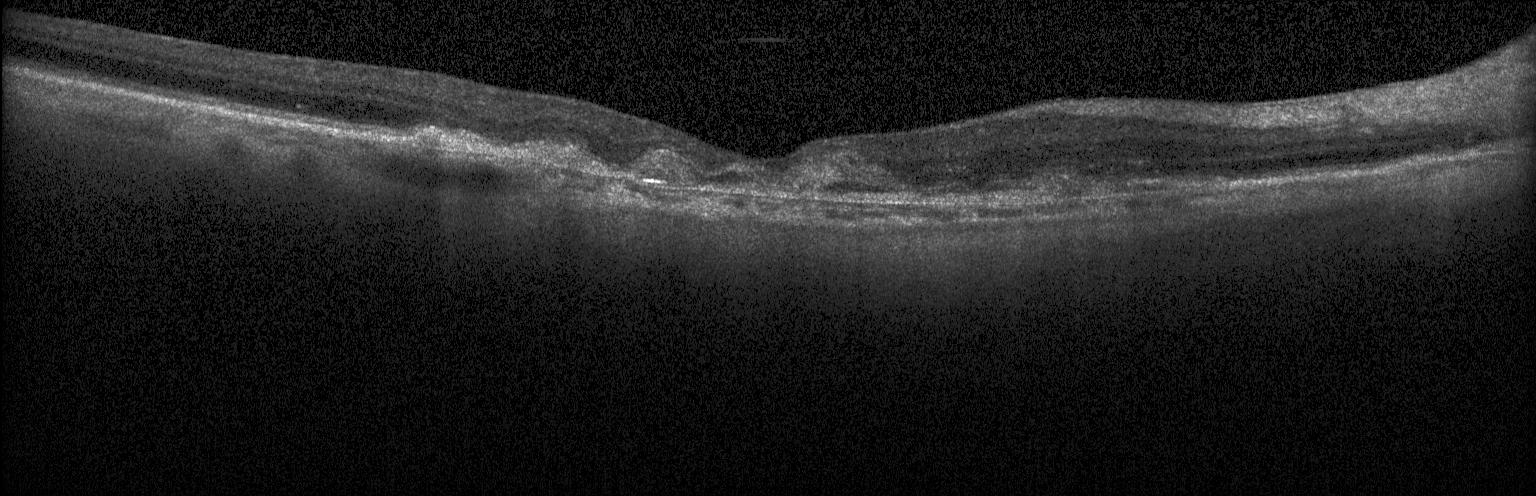
OCT B-scan. The scan shows a choroidal neovascular membrane.